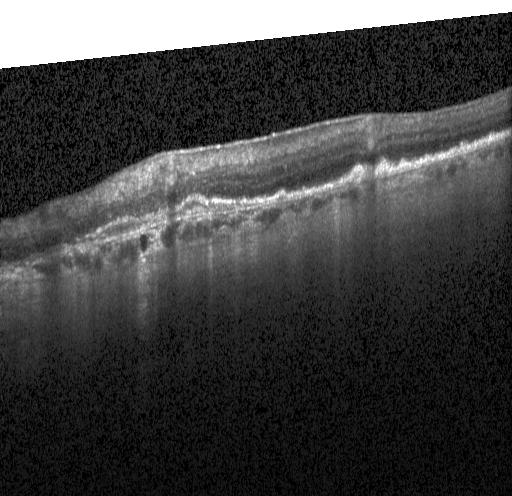

Through the macula. Optical coherence tomography scan. SD-OCT. Acquired on a Heidelberg Spectralis. The scan shows a choroidal neovascular membrane.